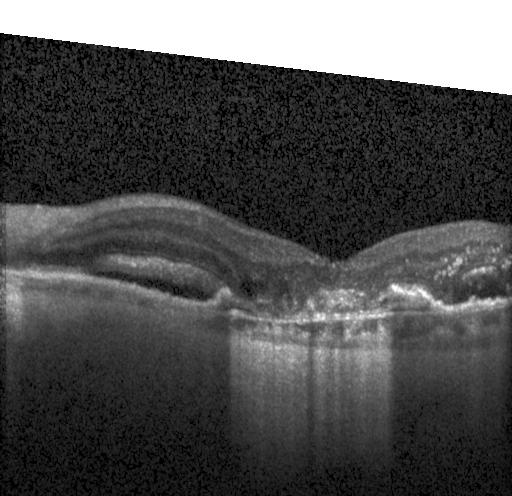
Finding: CNV.